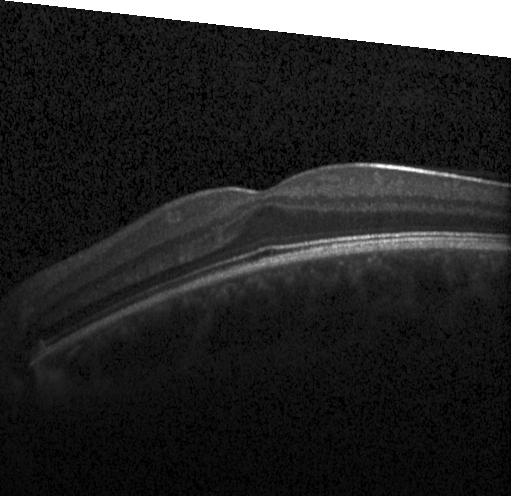
OCT finding: no evidence of choroidal neovascularization, diabetic macular edema, or drusen.